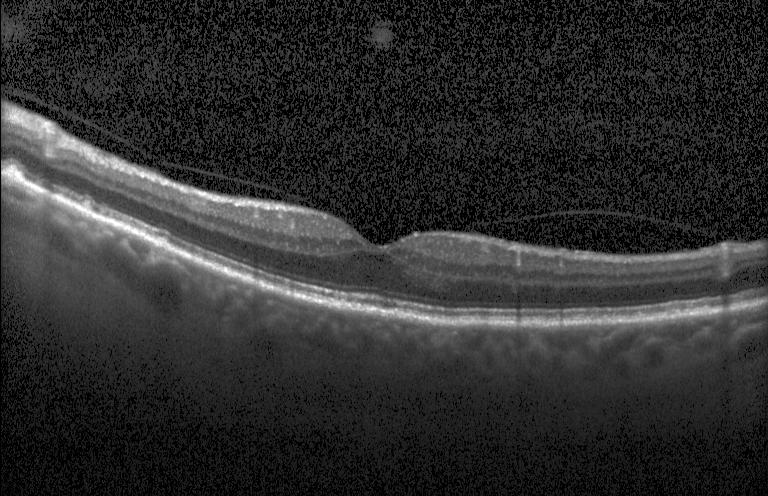 Diagnosis: no evidence of CNV, DME, or drusen.